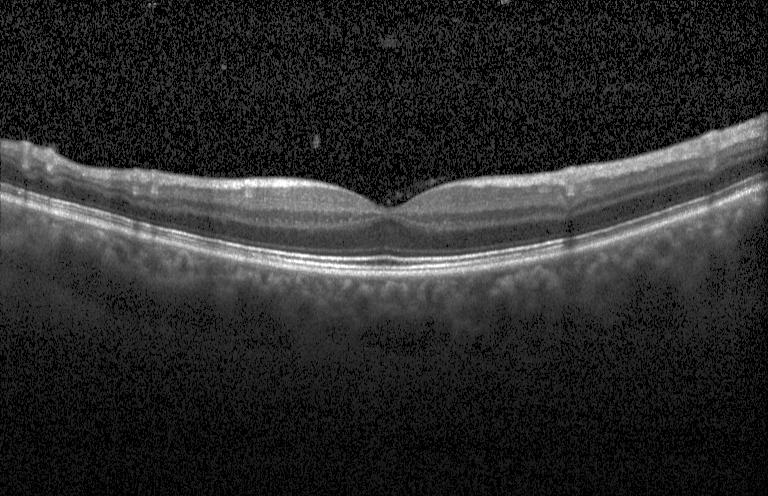

Finding: no evidence of CNV, DME, or drusen.